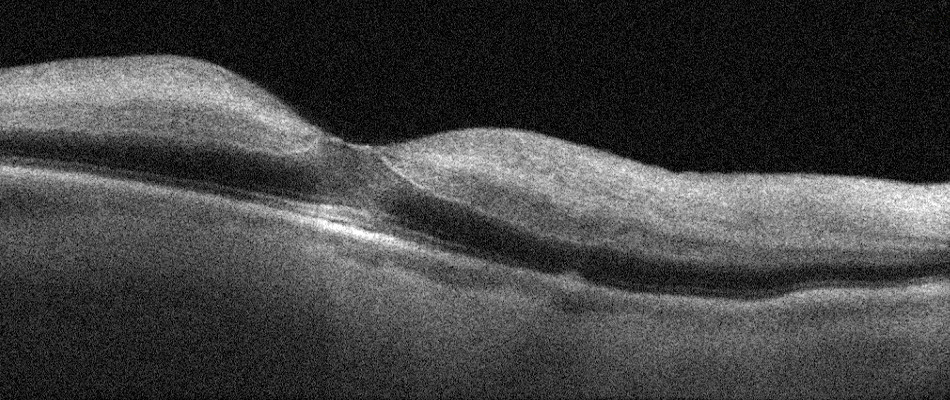

Macular OCT: retinal artery occlusion.